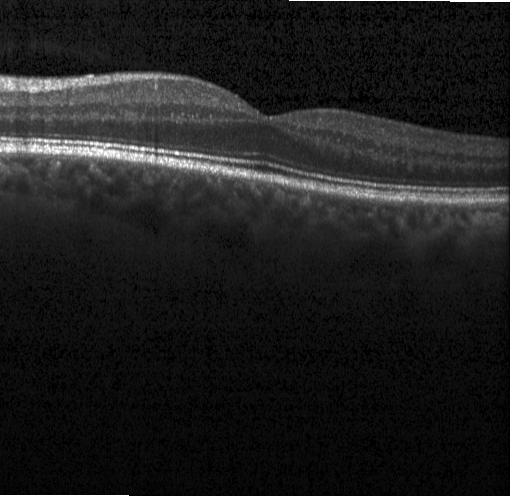 Optical coherence tomography B-scan, spectral-domain OCT
Impression: neither choroidal neovascularization, diabetic macular edema, nor drusen.